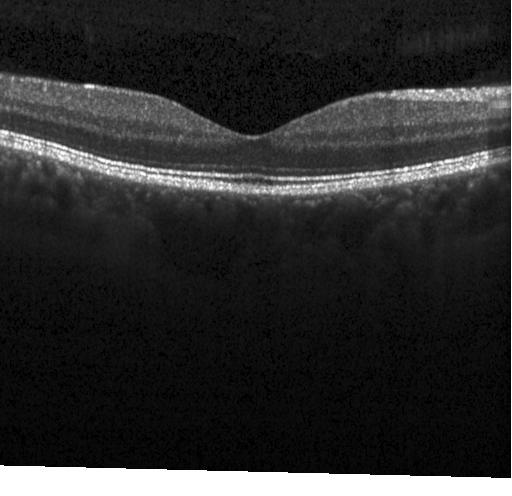 Heidelberg Spectralis · spectral-domain optical coherence tomography · centered on the fovea · retinal OCT B-scan — Diagnosis: no CNV, DME, or drusen.